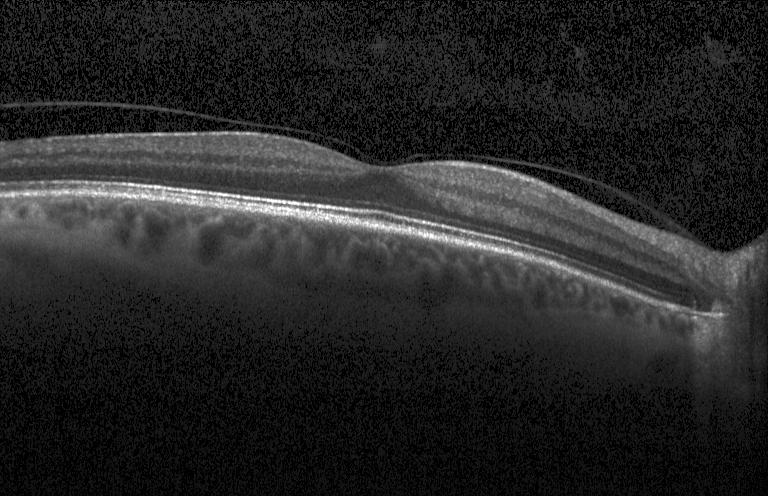

This B-scan demonstrates no choroidal neovascularization, diabetic macular edema, or drusen.